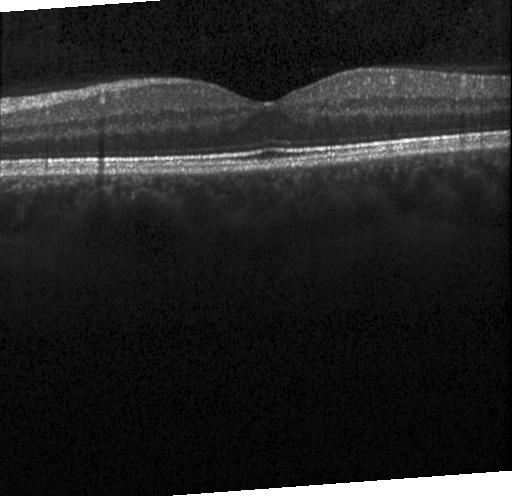
Impression: no CNV, no DME, and no drusen.